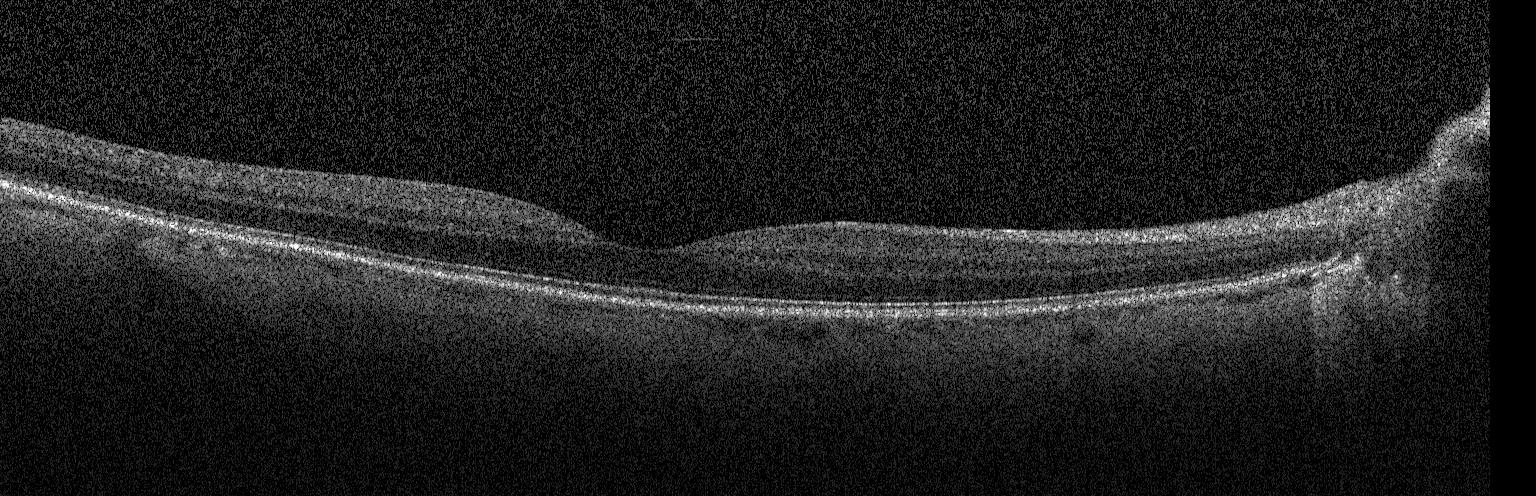
Retinal OCT cross-section. Impression: no evidence of CNV, DME, or drusen.